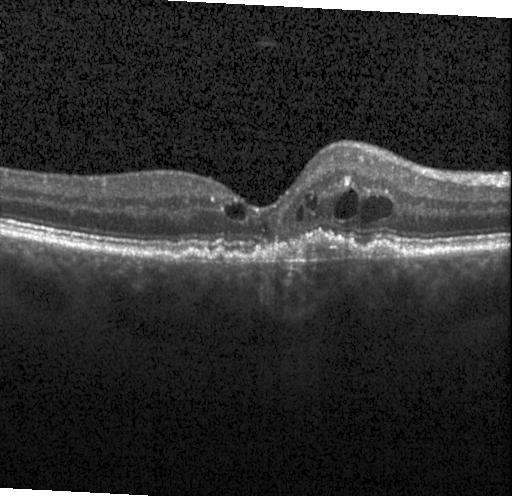 Retinal OCT cross-section showing a choroidal neovascular membrane.